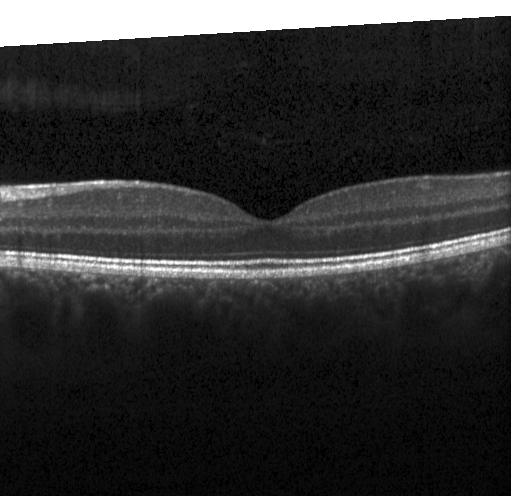
Finding: no evidence of choroidal neovascularization, diabetic macular edema, or drusen.